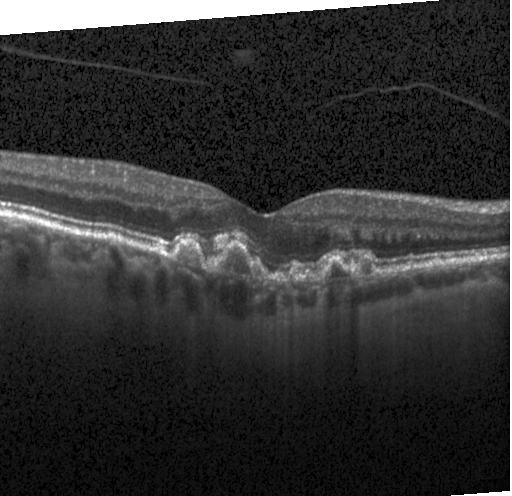 Macular OCT: CNV.